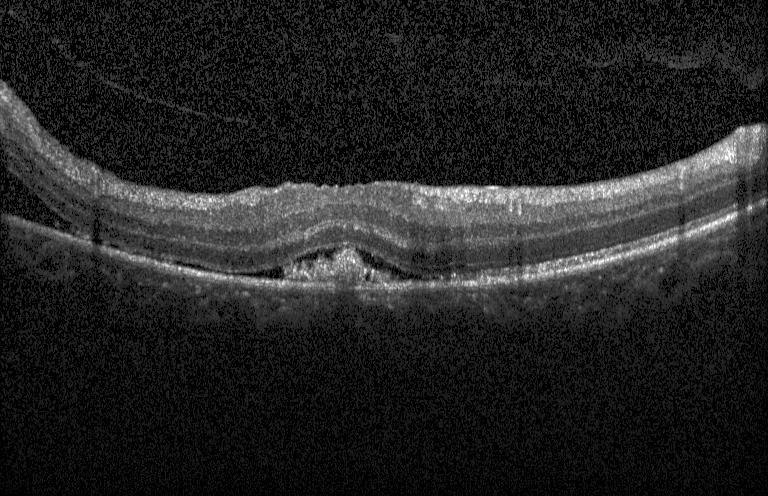
Instrument: Heidelberg Spectralis, OCT line scan — Assessment: choroidal neovascularization (CNV).